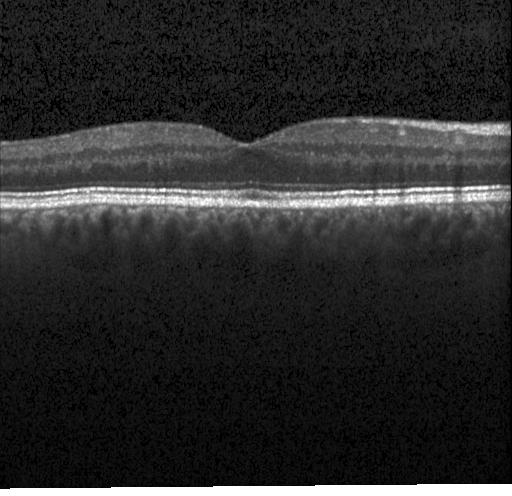

Optical coherence tomography B-scan; SD-OCT — Assessment: no choroidal neovascularization, diabetic macular edema, or drusen.